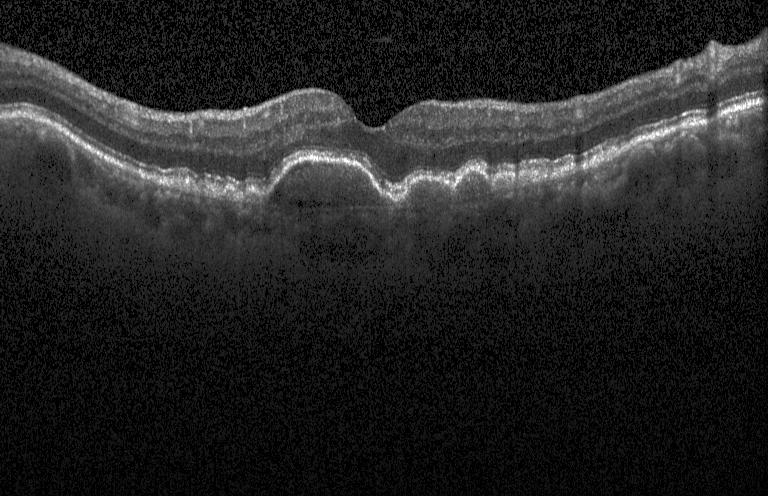

Assessment: drusen.